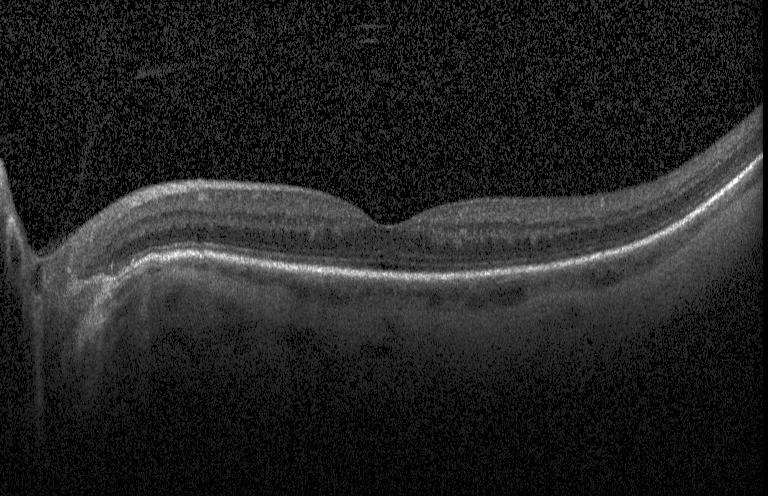

Instrument: Heidelberg Spectralis; optical coherence tomography scan — This B-scan demonstrates no choroidal neovascularization, no diabetic macular edema, and no drusen.